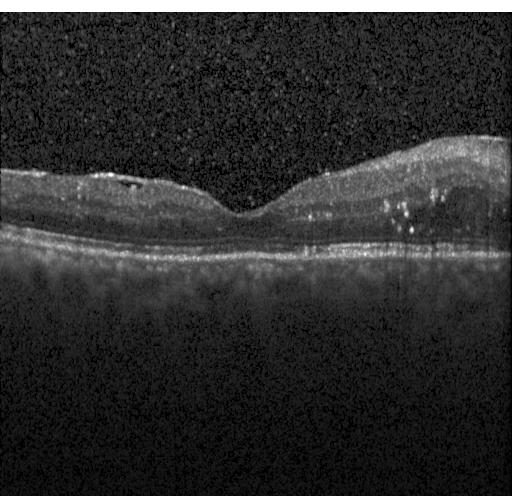
Macular OCT demonstrating diabetic macular edema.